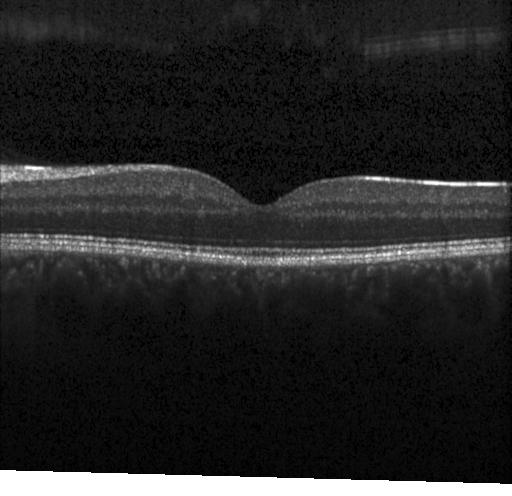 Impression: neither choroidal neovascularization, diabetic macular edema, nor drusen.